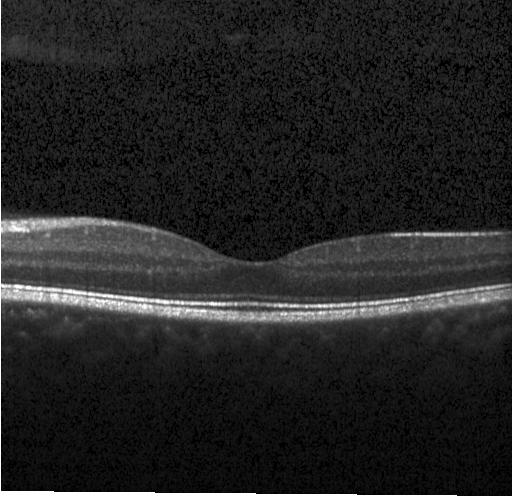

Acquired on a Heidelberg Spectralis. OCT line scan. SD-OCT — Diagnosis: no evidence of choroidal neovascularization, diabetic macular edema, or drusen.